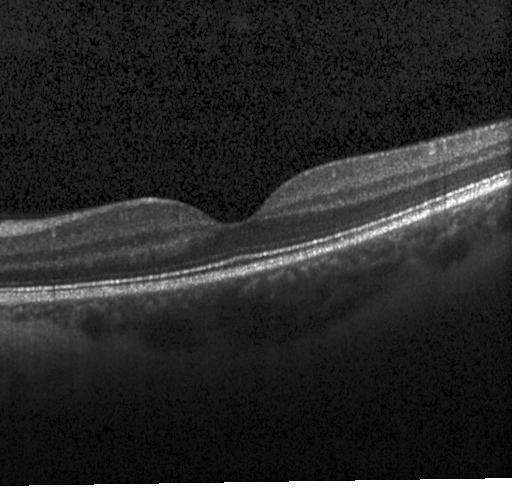 Spectral-domain optical coherence tomography · retinal OCT B-scan. Diagnosis: no evidence of choroidal neovascularization, diabetic macular edema, or drusen.